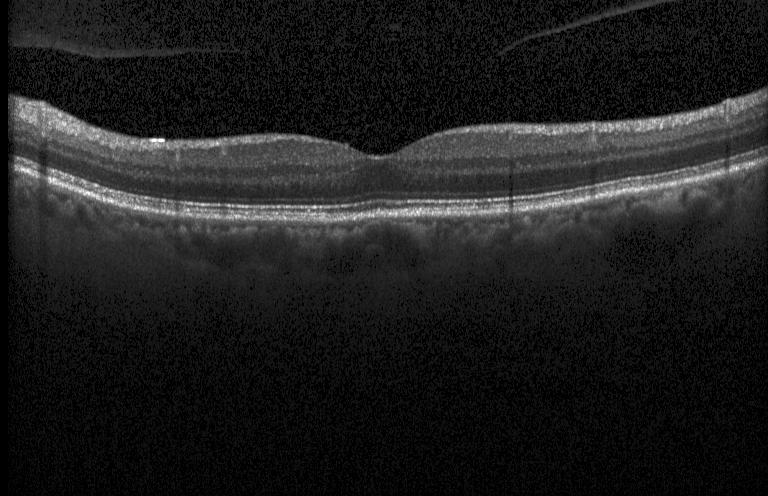 Retinal OCT cross-section showing no choroidal neovascularization, no diabetic macular edema, and no drusen.